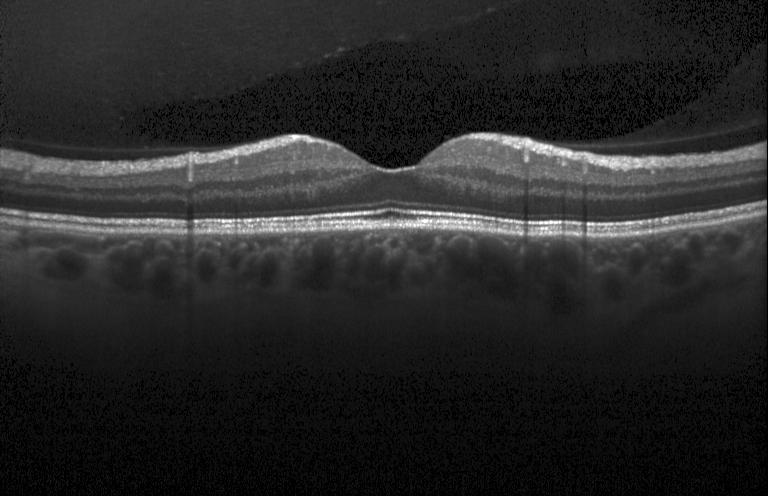 Dx: no CNV, no DME, and no drusen.